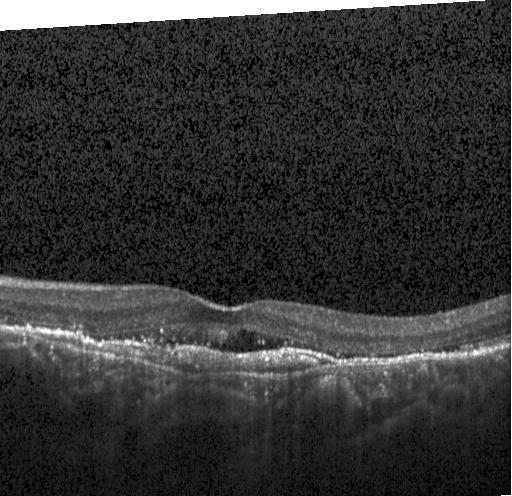

Spectral-domain optical coherence tomography. Horizontal scan through the fovea. Optical coherence tomography scan. Heidelberg Spectralis.
Finding: CNV.